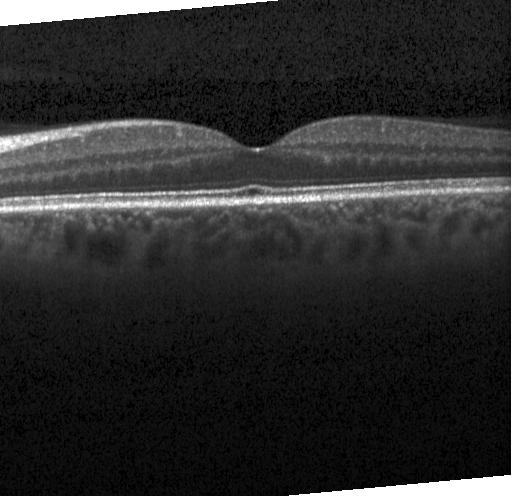 Retinal OCT cross-section
Impression: no evidence of CNV, DME, or drusen.